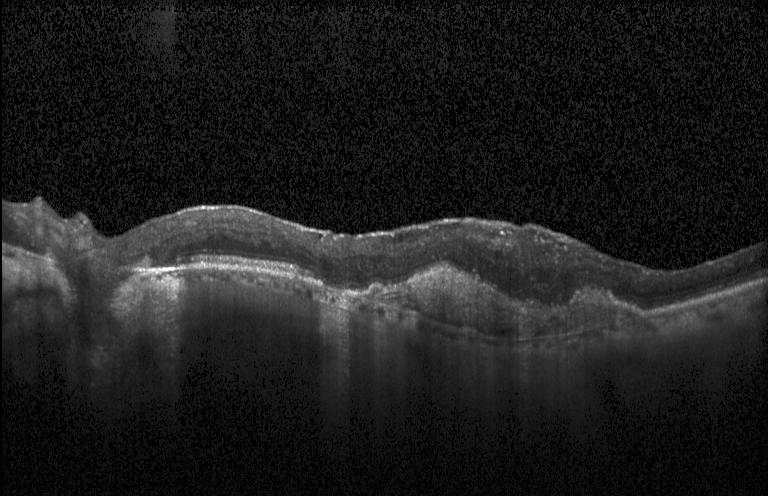
Retinal OCT B-scan · fovea-centered — Diagnosis: choroidal neovascularization (CNV).